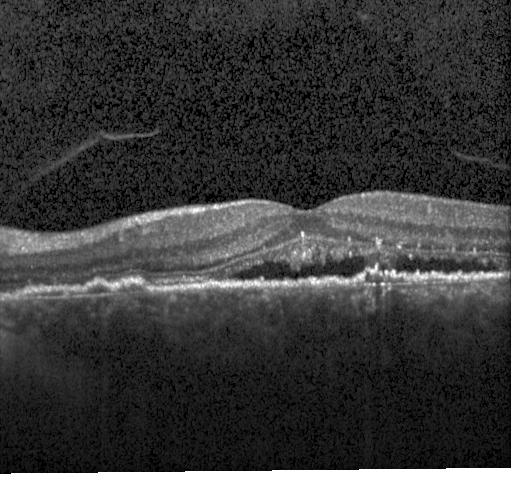
Optical coherence tomography scan; Heidelberg Spectralis OCT system
Finding: a choroidal neovascular membrane.